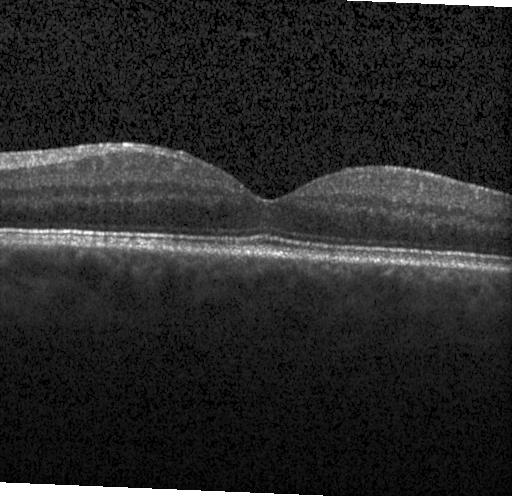 Spectral-domain OCT; Heidelberg Spectralis OCT system; OCT B-scan; fovea-centered
Diagnosis: no choroidal neovascularization, no diabetic macular edema, and no drusen.